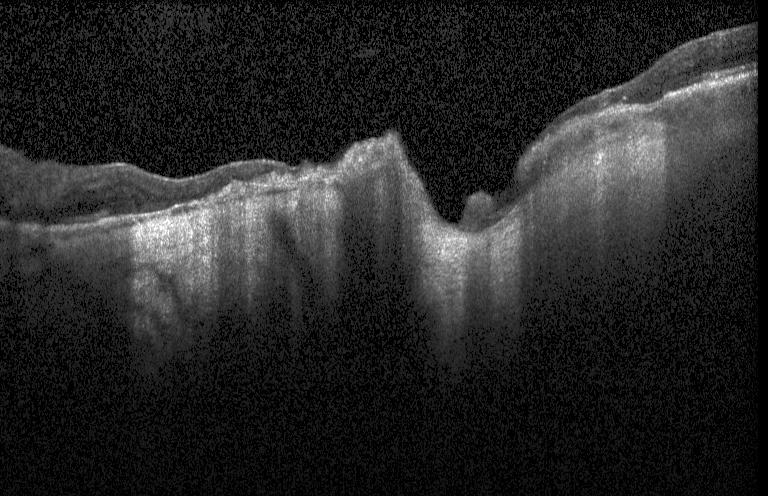

Spectral-domain OCT B-scan: a choroidal neovascular membrane.